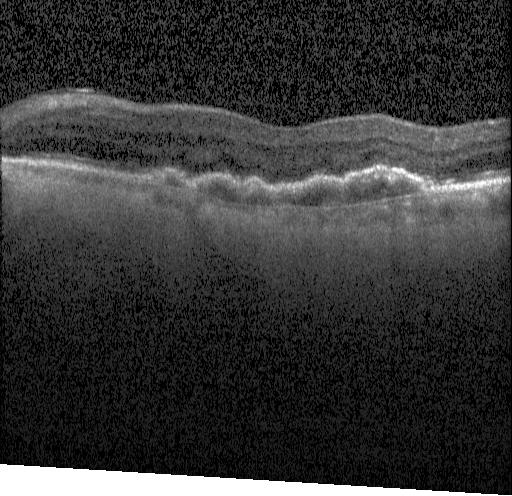
Diagnosis: a choroidal neovascular membrane.